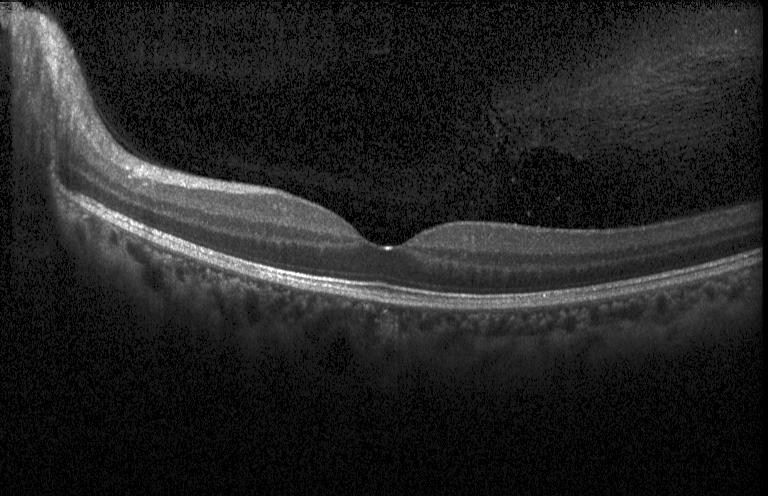

Optical coherence tomography scan. SD-OCT.
Finding: no choroidal neovascularization, no diabetic macular edema, and no drusen.